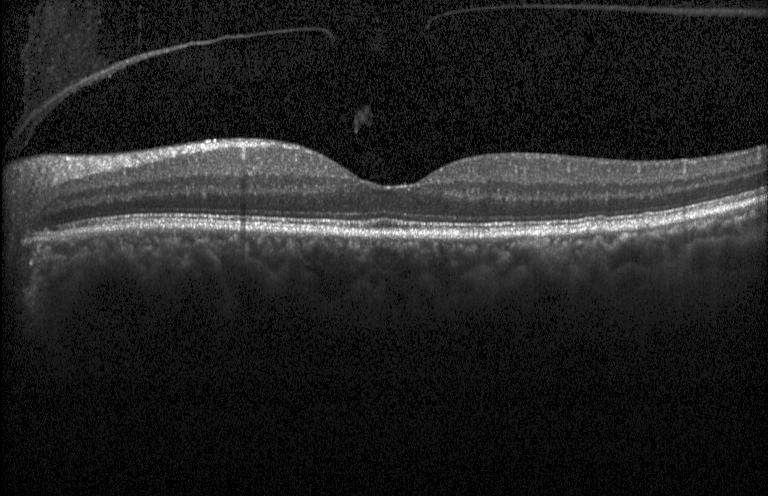
Optical coherence tomography B-scan · instrument: Heidelberg Spectralis. Assessment: no evidence of choroidal neovascularization, diabetic macular edema, or drusen.